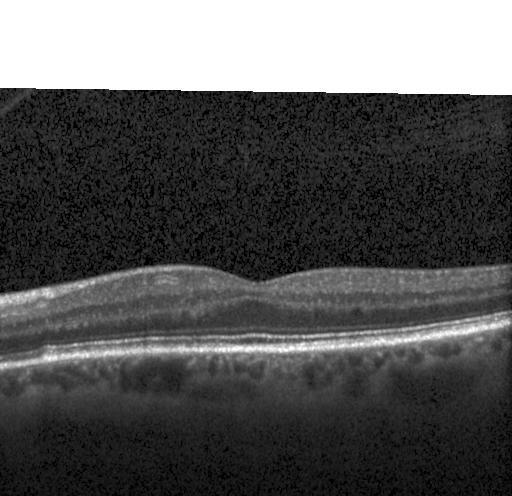 The scan shows neither choroidal neovascularization, diabetic macular edema, nor drusen.